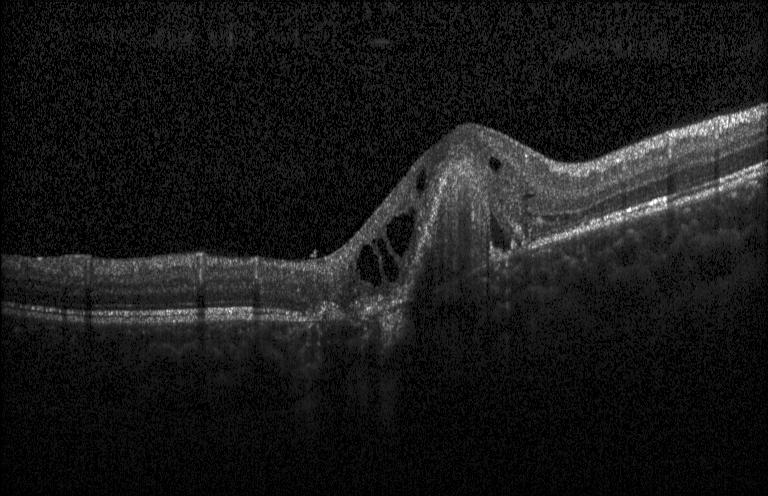 Diagnosis: choroidal neovascularization.